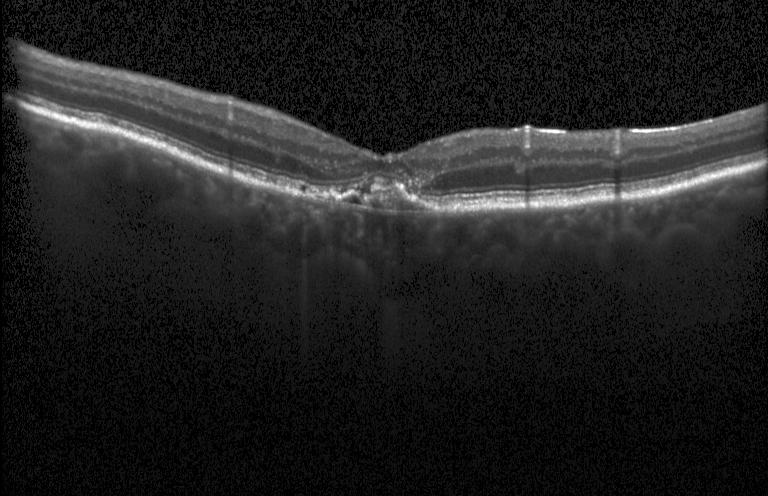

OCT line scan. Spectral-domain optical coherence tomography.
Dx: a choroidal neovascular membrane.